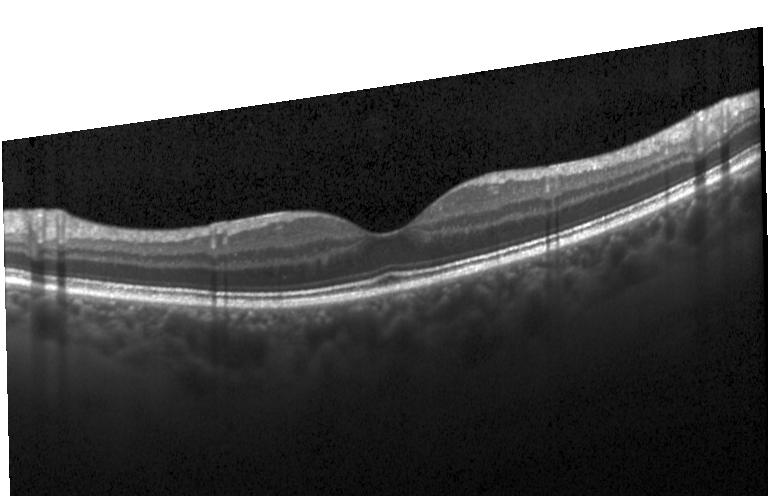

OCT B-scan. Impression: no CNV, no DME, and no drusen.